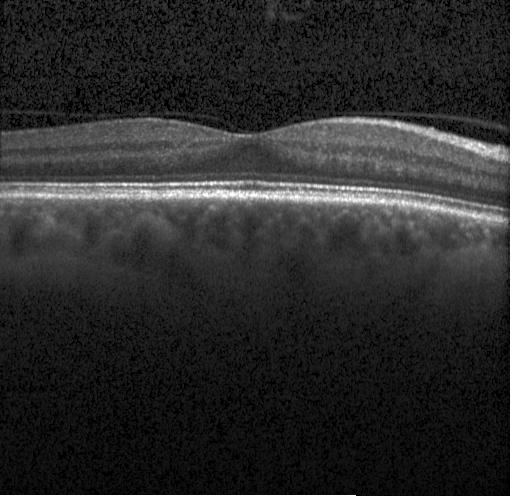

Centered on the fovea · retinal OCT B-scan — This B-scan demonstrates neither CNV, DME, nor drusen.